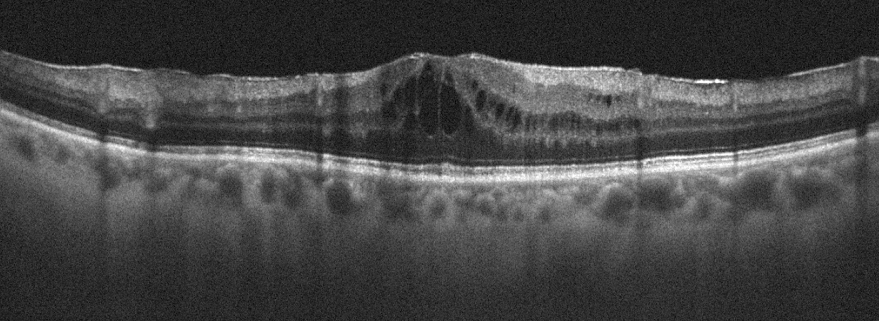 Impression: diabetic macular edema (DME).